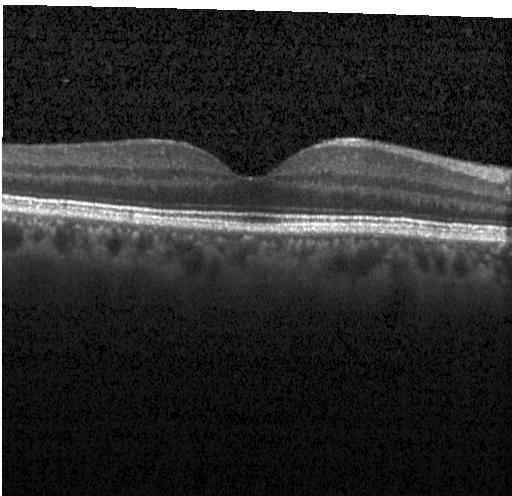
Spectral-domain OCT B-scan: no choroidal neovascularization, diabetic macular edema, or drusen.